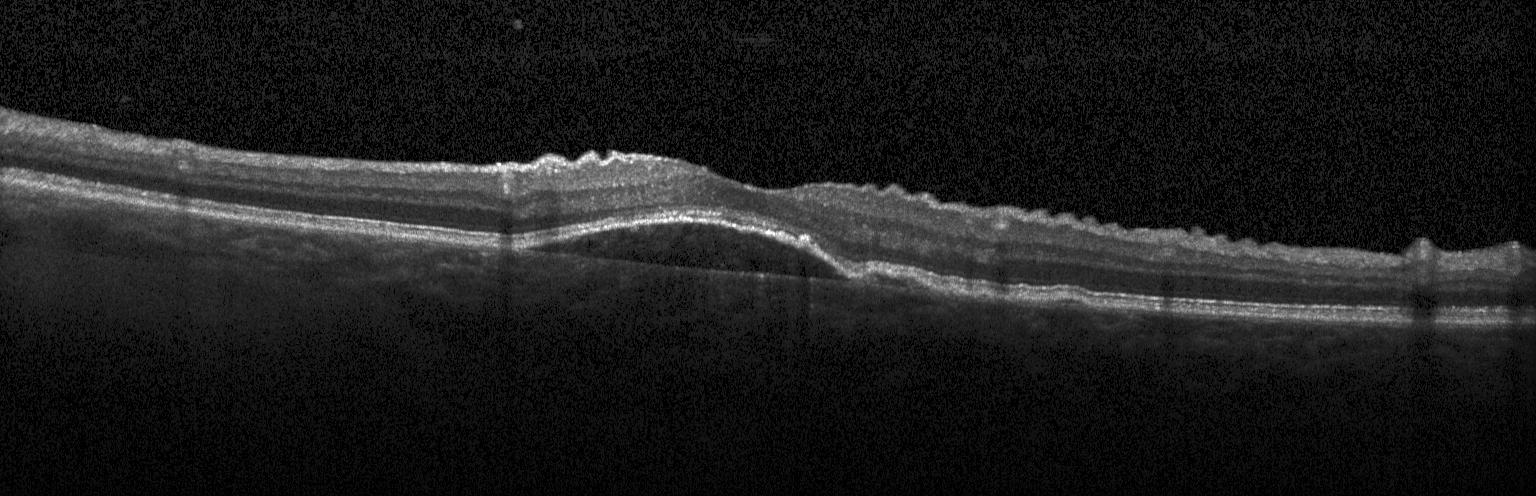 Finding: a choroidal neovascular membrane.